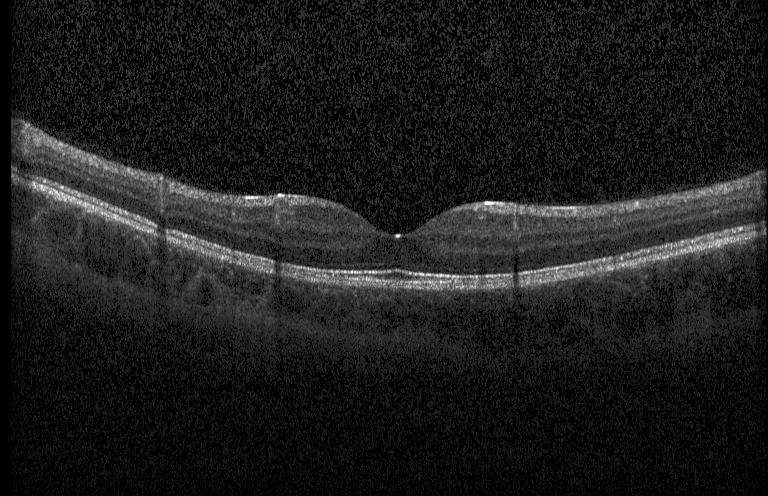 Macular OCT: neither choroidal neovascularization, diabetic macular edema, nor drusen.